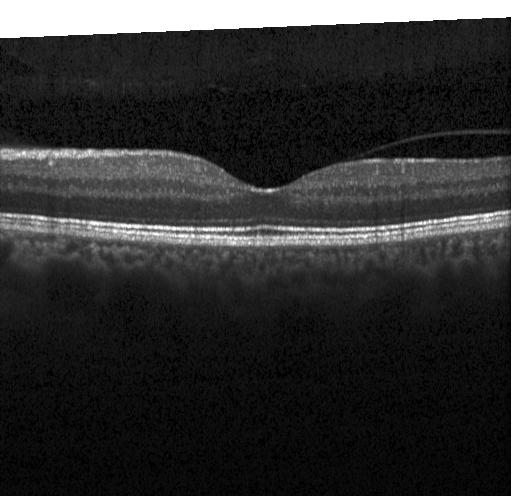 Retinal OCT B-scan.
Neither choroidal neovascularization, diabetic macular edema, nor drusen.